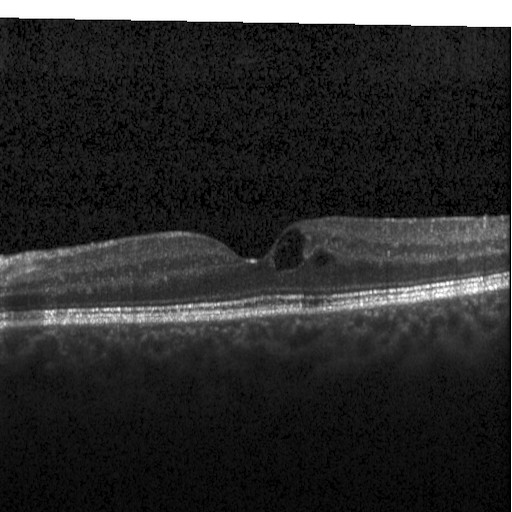
Impression: DME.